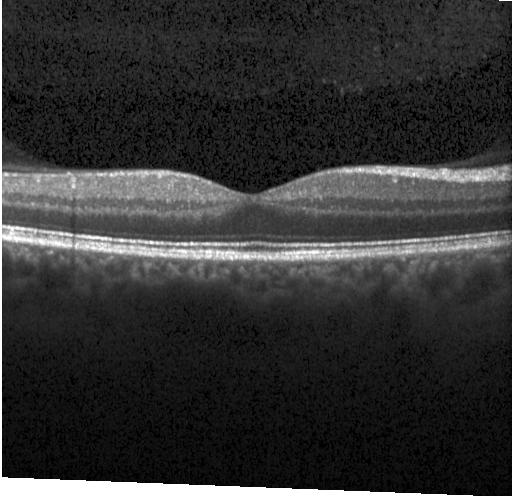
Spectral-domain OCT, optical coherence tomography scan, centered on the fovea
Impression: no CNV, DME, or drusen.